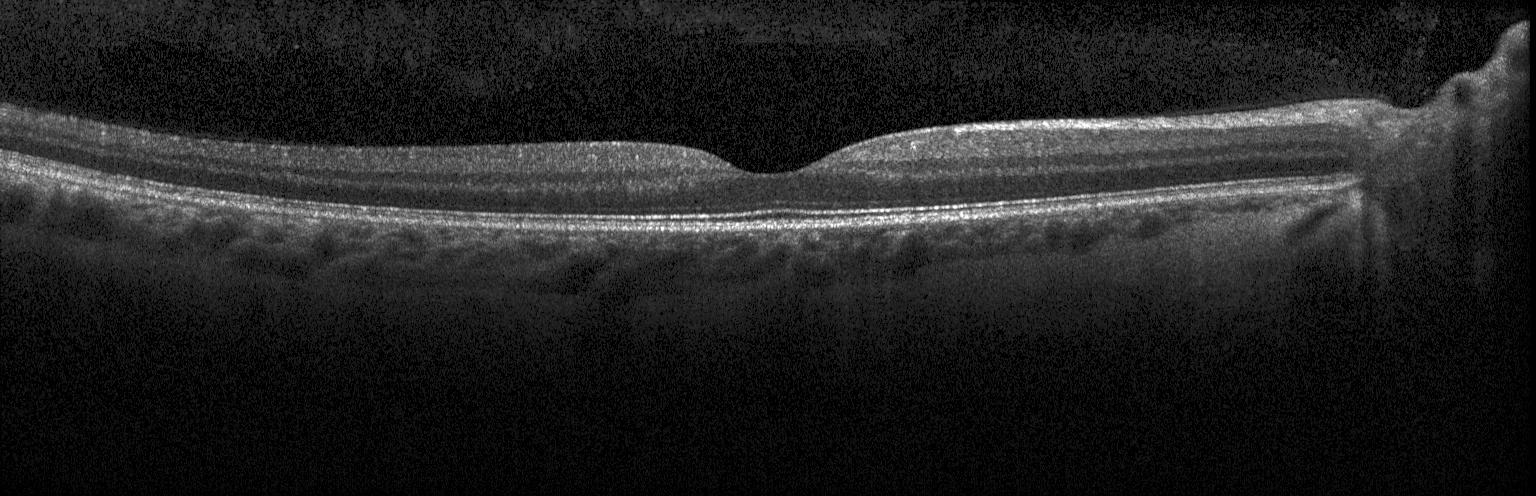

OCT scan showing no choroidal neovascularization, no diabetic macular edema, and no drusen.